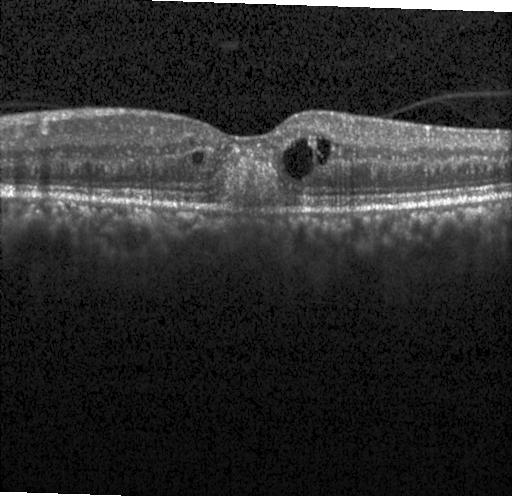 Retinal OCT B-scan — Finding: CNV.